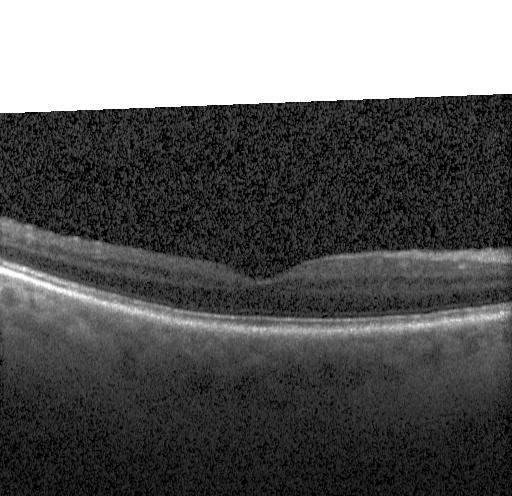 Spectral-domain optical coherence tomography. Heidelberg Spectralis OCT system. Retinal OCT B-scan. Fovea-centered — The scan shows no CNV, DME, or drusen.